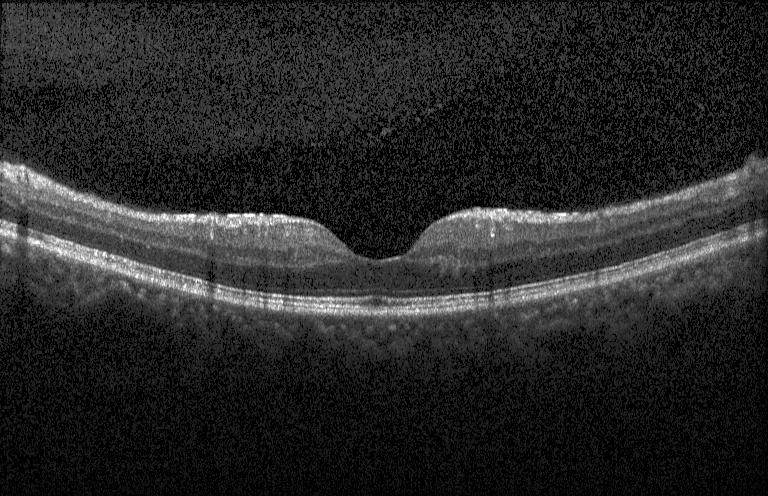
Optical coherence tomography B-scan, through the macula, spectral-domain optical coherence tomography, instrument: Heidelberg Spectralis — Impression: no evidence of choroidal neovascularization, diabetic macular edema, or drusen.